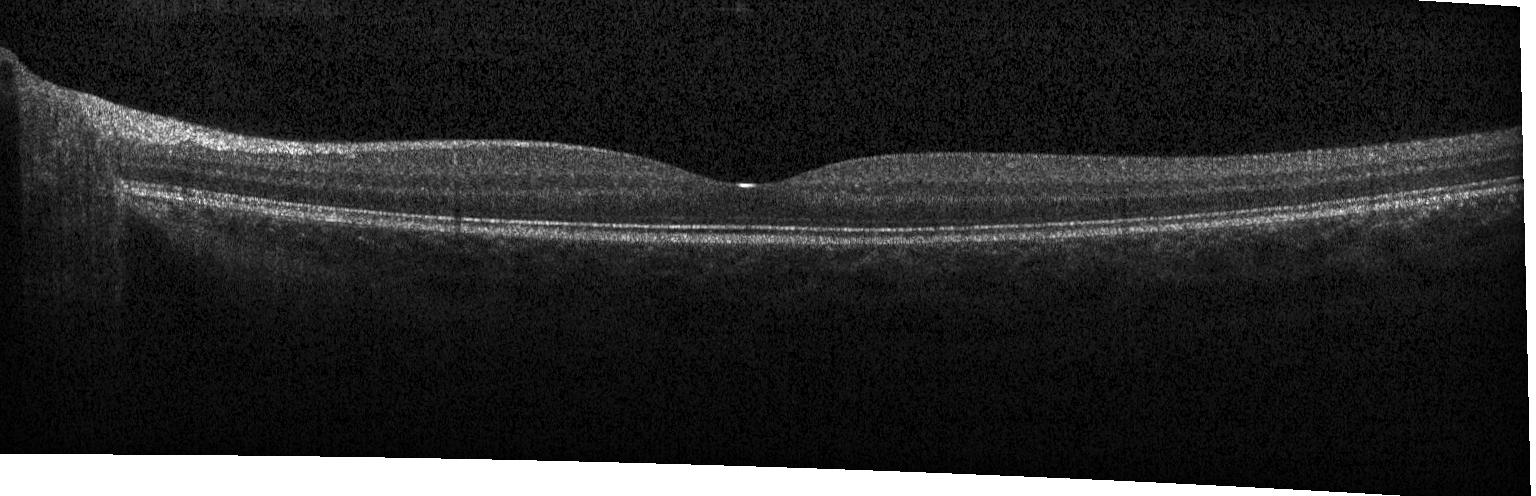
This B-scan demonstrates no CNV, DME, or drusen.